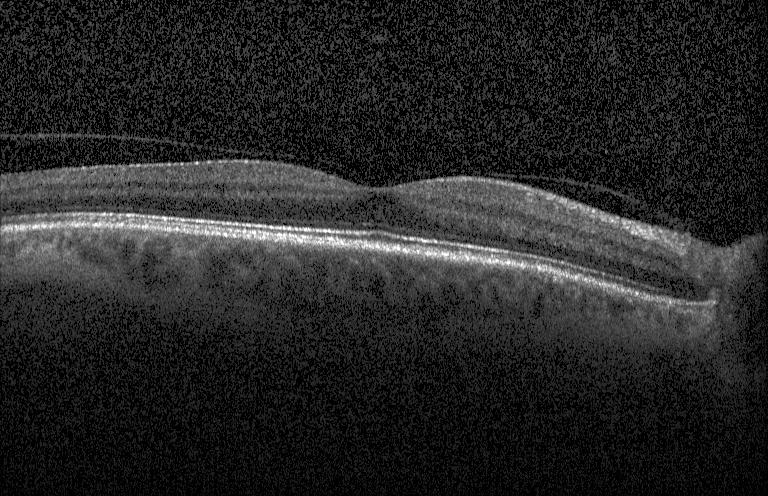
Macular scan; acquired on a Heidelberg Spectralis; retinal OCT cross-section; spectral-domain optical coherence tomography — Neither choroidal neovascularization, diabetic macular edema, nor drusen.